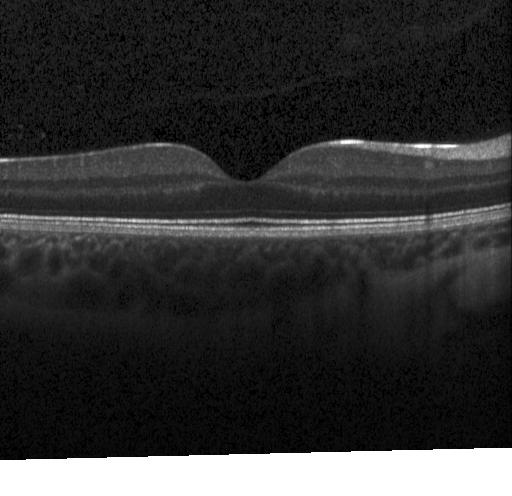 OCT scan showing no CNV, no DME, and no drusen.